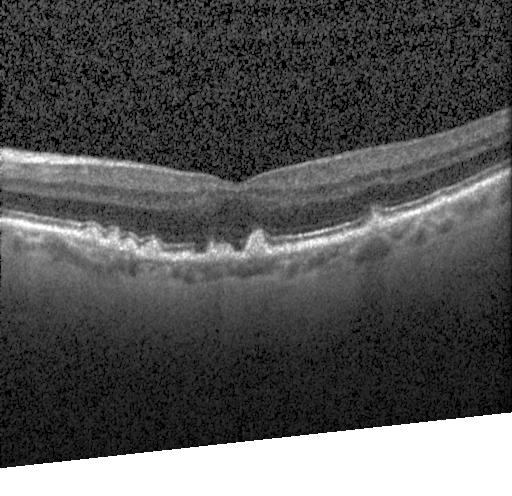
Retinal OCT cross-section · spectral-domain optical coherence tomography. This B-scan demonstrates multiple drusen.